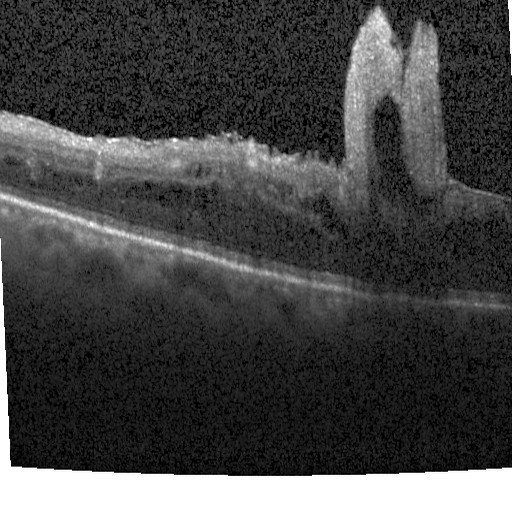 Spectral-domain optical coherence tomography. OCT line scan
Dx: DME.